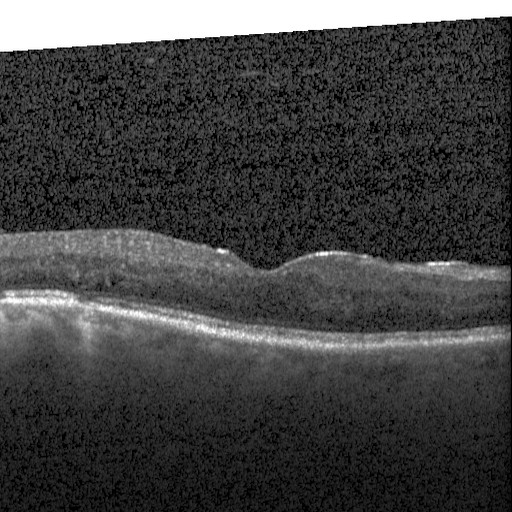
OCT line scan. Instrument: Heidelberg Spectralis. Spectral-domain OCT
The scan shows diabetic macular edema.